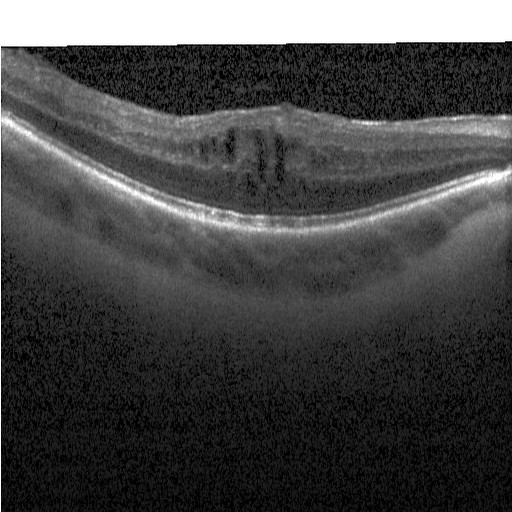
Heidelberg Spectralis; retinal OCT cross-section; macular scan. The scan shows DME.